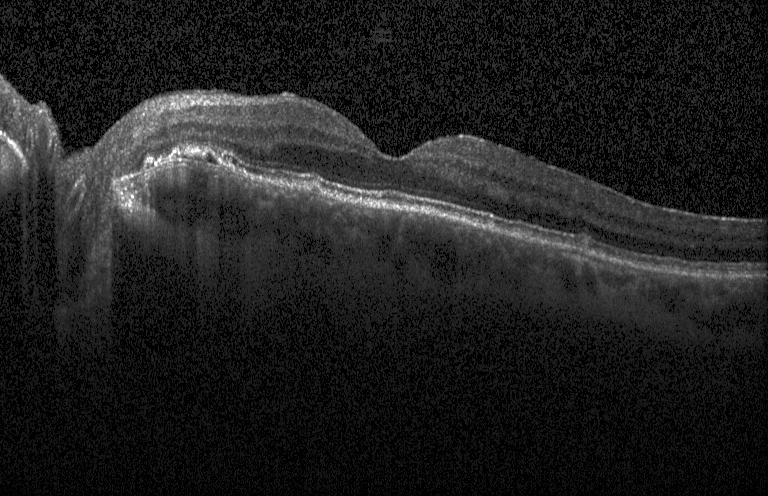

Acquired on a Heidelberg Spectralis, macular scan, spectral-domain optical coherence tomography, optical coherence tomography scan. Macular OCT: drusen.